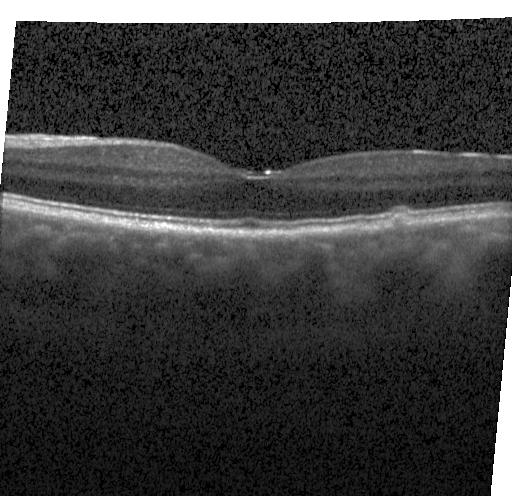

Spectral-domain OCT B-scan: drusen.